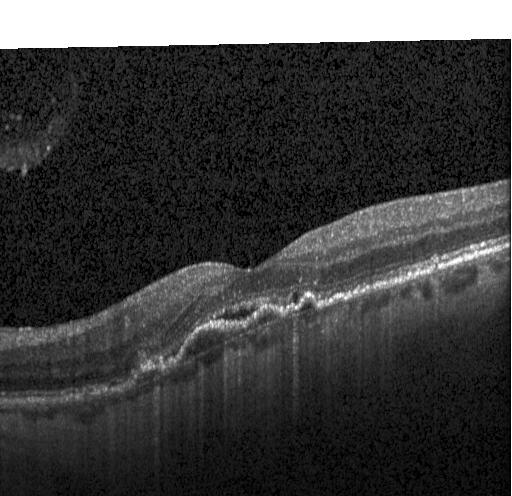 Diagnosis: a choroidal neovascular membrane.